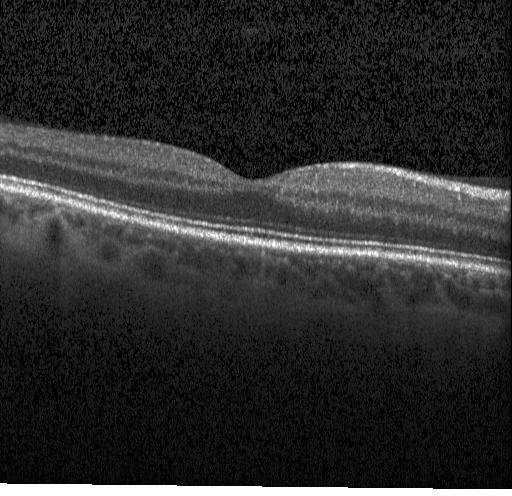
Diagnosis: neither choroidal neovascularization, diabetic macular edema, nor drusen.